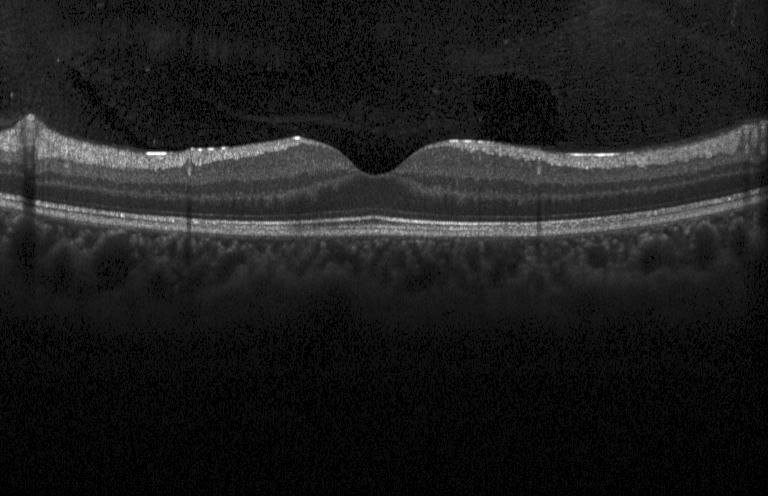 Heidelberg Spectralis OCT system; spectral-domain optical coherence tomography; optical coherence tomography scan; centered on the fovea. Finding: no evidence of choroidal neovascularization, diabetic macular edema, or drusen.